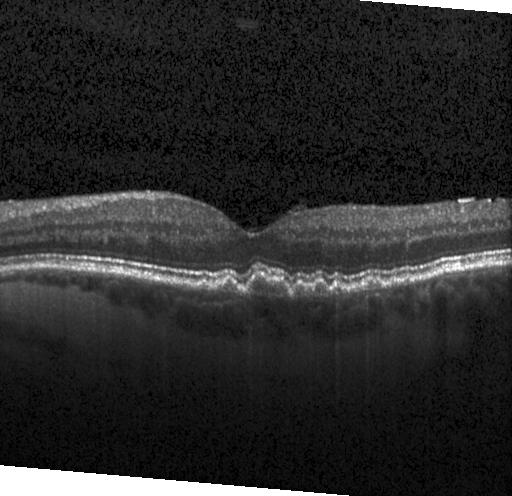
Spectral-domain OCT; OCT line scan. Diagnosis: drusen.